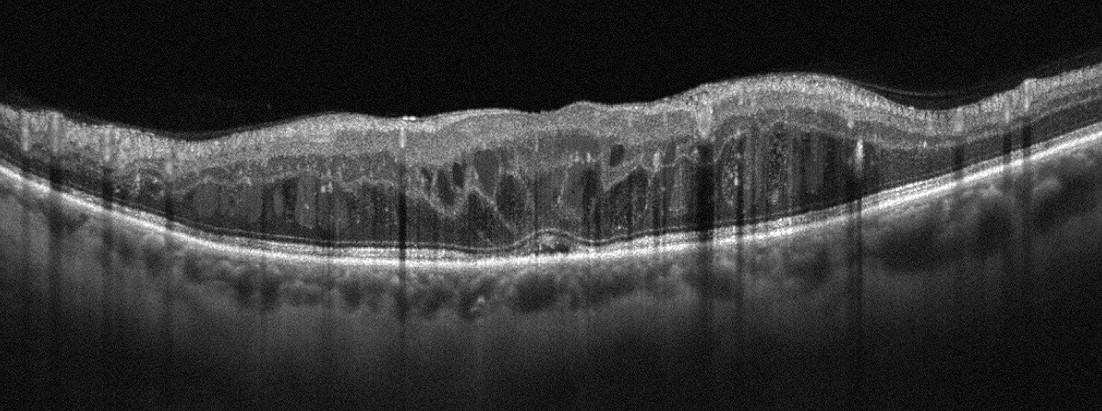 Instrument: Optovue Avanti RTVue XR. Retinal OCT cross-section.
Impression: diabetic macular edema.